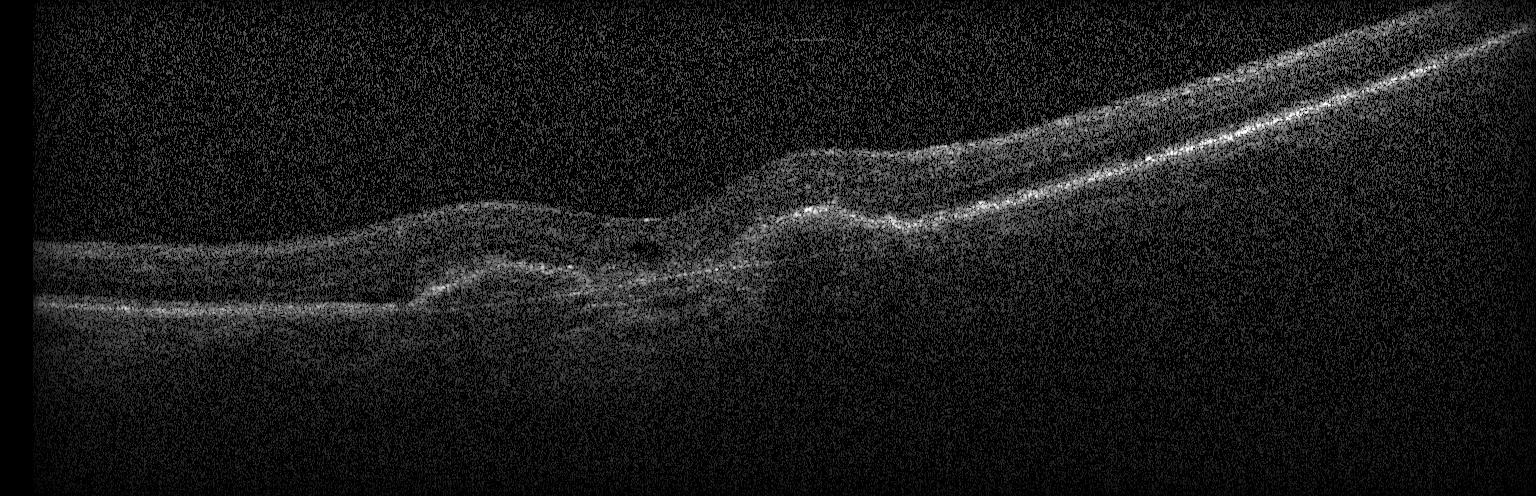
Finding: a choroidal neovascular membrane.